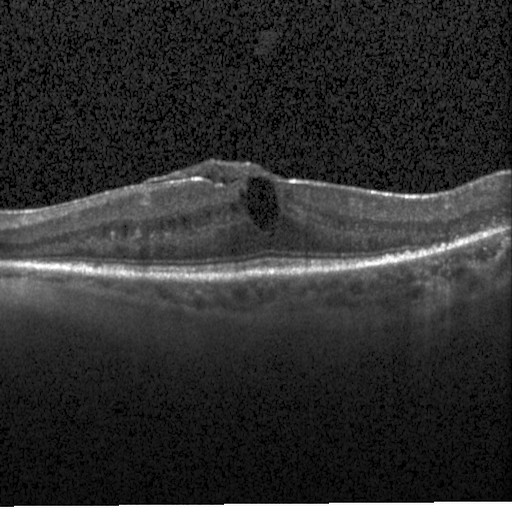
Optical coherence tomography B-scan.
Dx: diabetic macular edema.